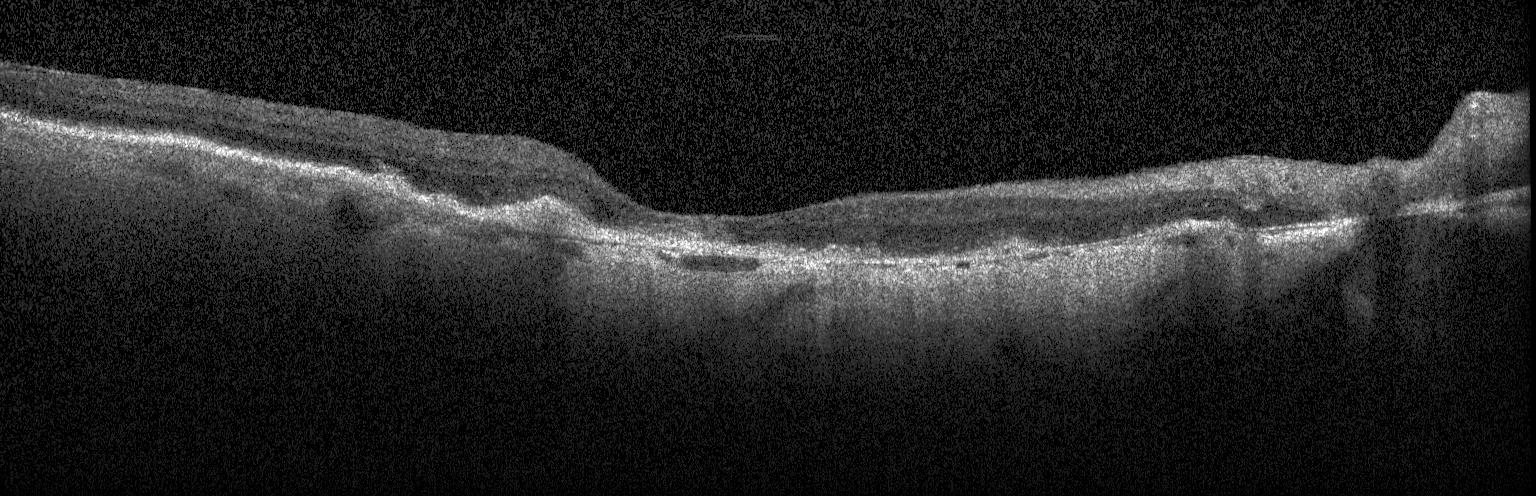

Impression: choroidal neovascularization.